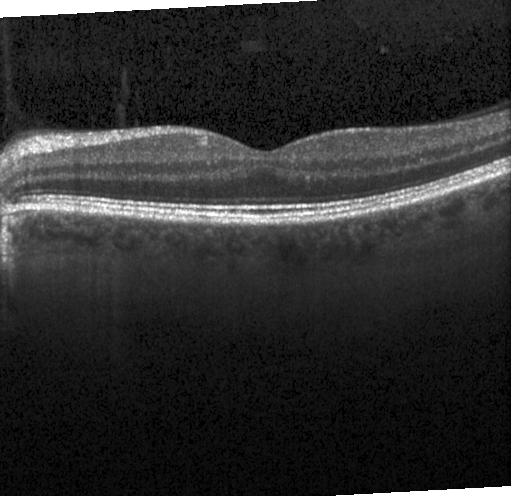 Heidelberg Spectralis OCT system. OCT line scan
This B-scan demonstrates no evidence of CNV, DME, or drusen.